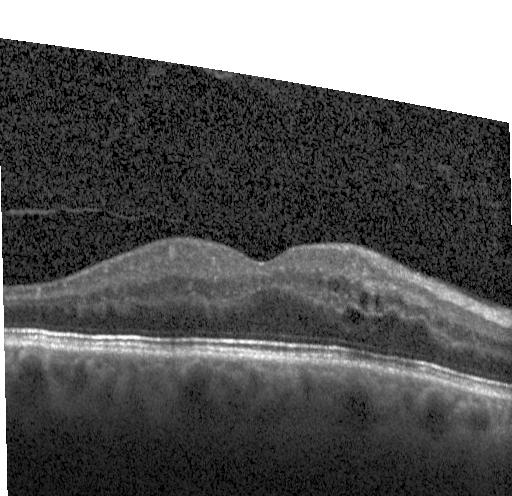

OCT scan showing DME.